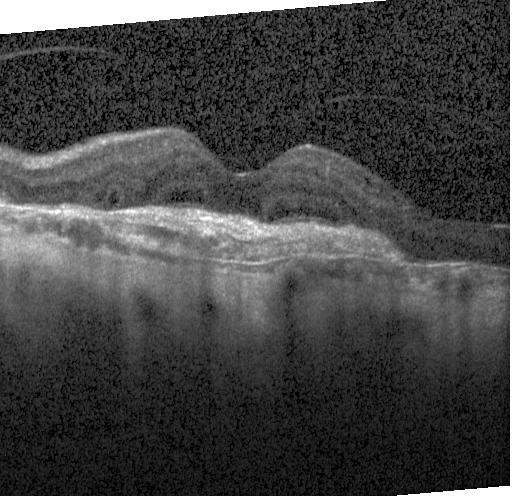

Retinal OCT cross-section — Finding: a choroidal neovascular membrane.